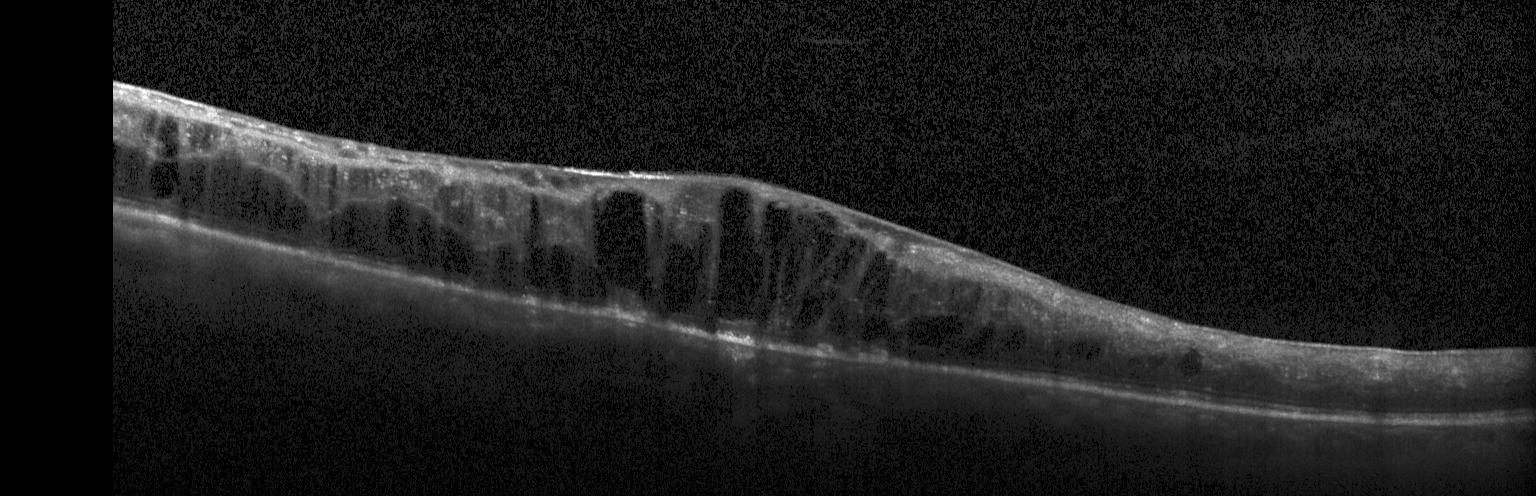

Assessment: diabetic macular edema.